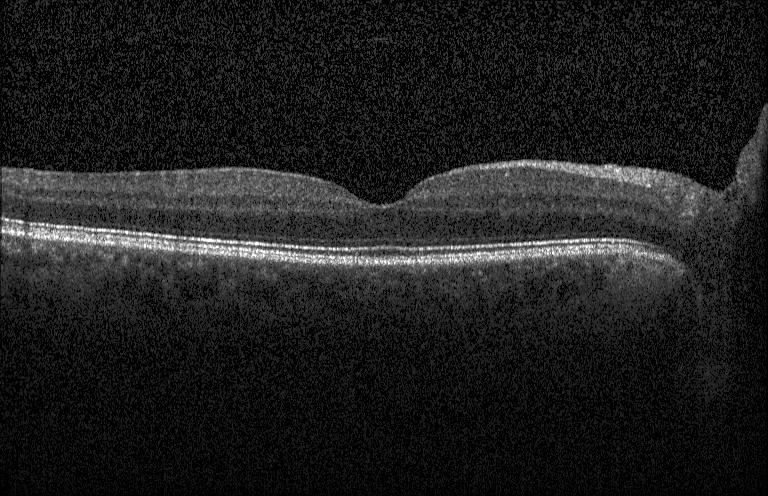

Through the macula; instrument: Heidelberg Spectralis; optical coherence tomography scan. Finding: no choroidal neovascularization, no diabetic macular edema, and no drusen.